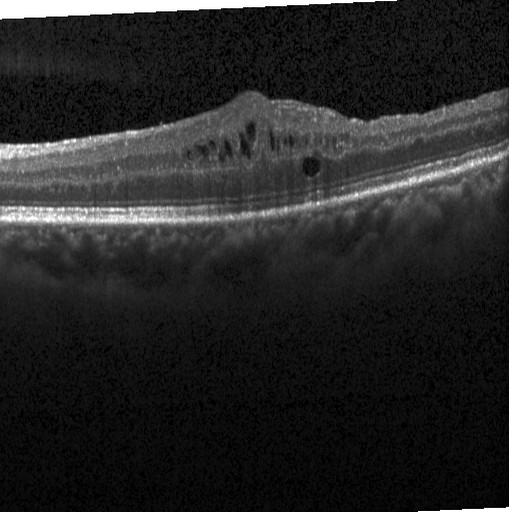 Instrument: Heidelberg Spectralis. Macular scan. Optical coherence tomography scan. SD-OCT
DME.